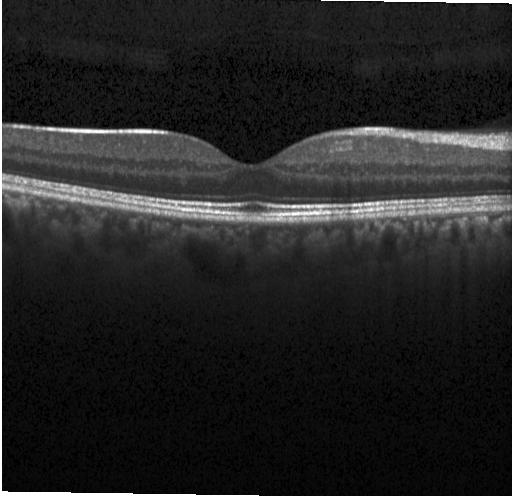
OCT B-scan — Macular OCT: no evidence of choroidal neovascularization, diabetic macular edema, or drusen.